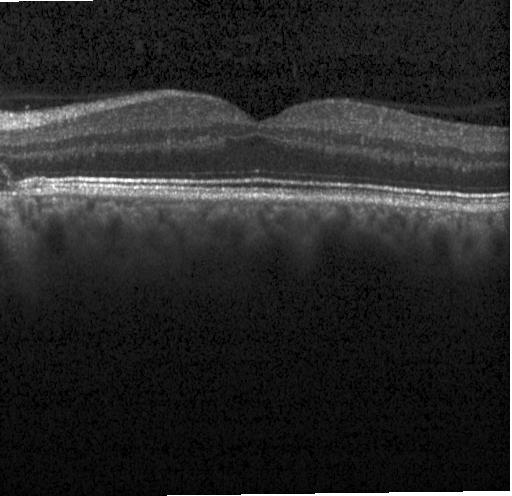 Spectral-domain optical coherence tomography; optical coherence tomography B-scan.
Impression: no choroidal neovascularization, diabetic macular edema, or drusen.